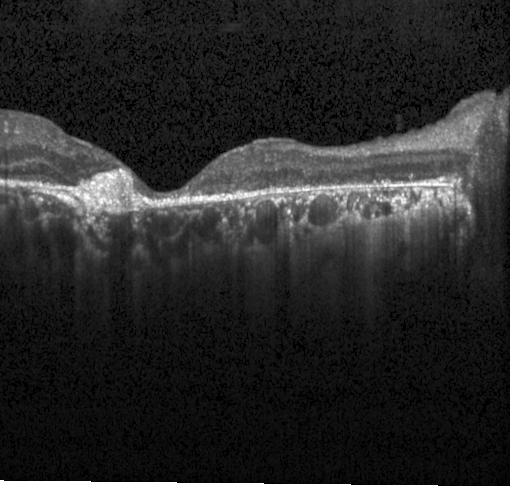 Horizontal scan through the fovea, spectral-domain OCT, retinal OCT B-scan.
A choroidal neovascular membrane.